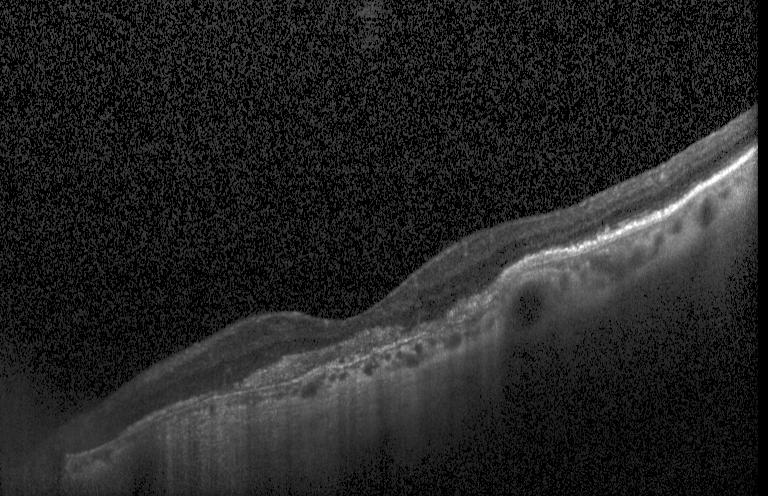

Through the macula, Heidelberg Spectralis, spectral-domain OCT, optical coherence tomography B-scan. This B-scan demonstrates choroidal neovascularization.